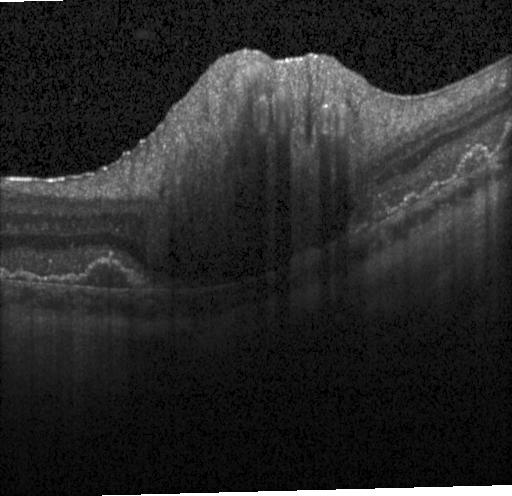

Acquired on a Heidelberg Spectralis. Optical coherence tomography scan
Diagnosis: a choroidal neovascular membrane.